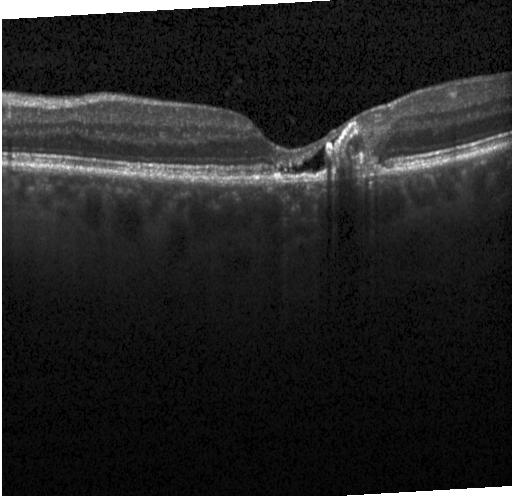 OCT line scan.
OCT finding: a choroidal neovascular membrane.